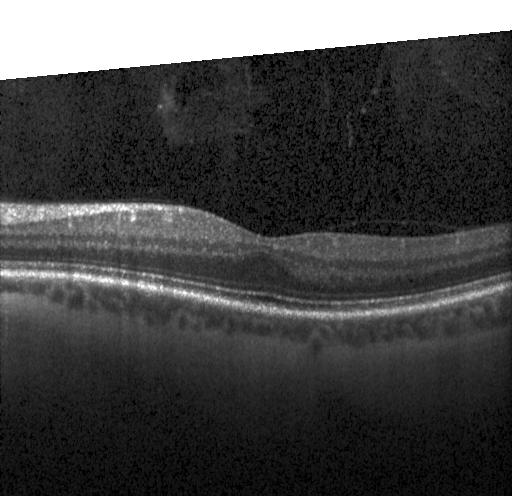

Optical coherence tomography scan. Spectral-domain optical coherence tomography. Instrument: Heidelberg Spectralis.
Impression: neither choroidal neovascularization, diabetic macular edema, nor drusen.